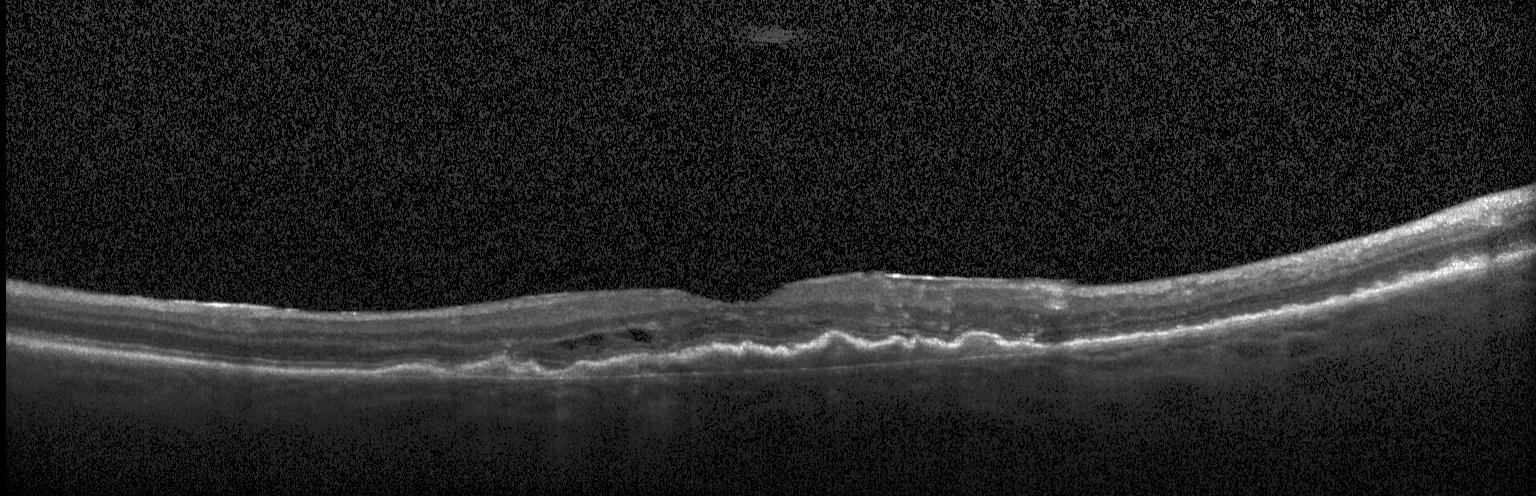
Horizontal scan through the fovea; retinal OCT B-scan; Heidelberg Spectralis OCT system. Impression: a choroidal neovascular membrane.